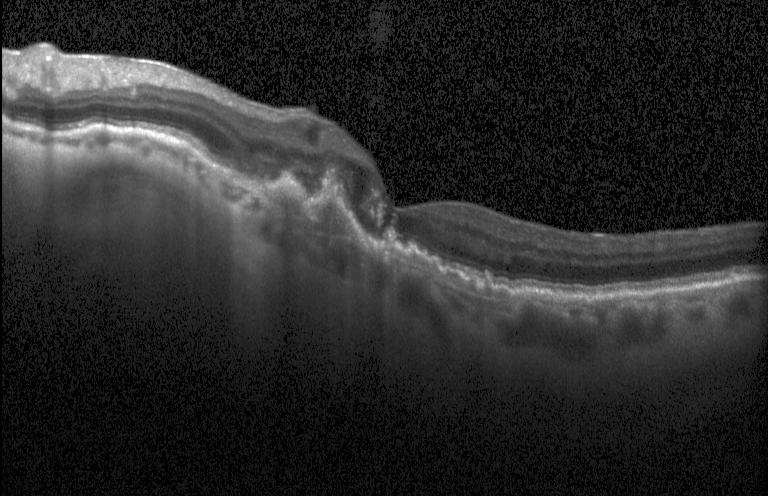
Macular OCT demonstrating choroidal neovascularization.